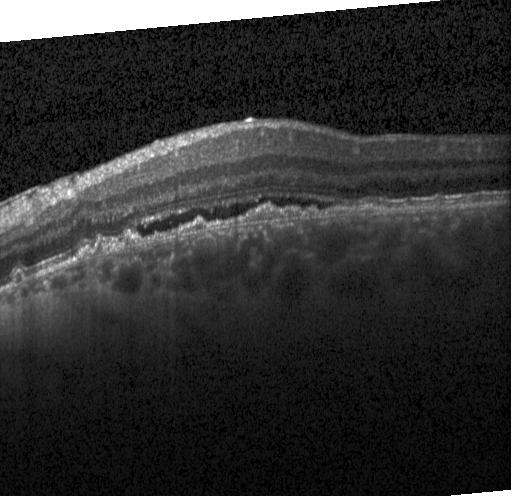 Macular OCT demonstrating a choroidal neovascular membrane.